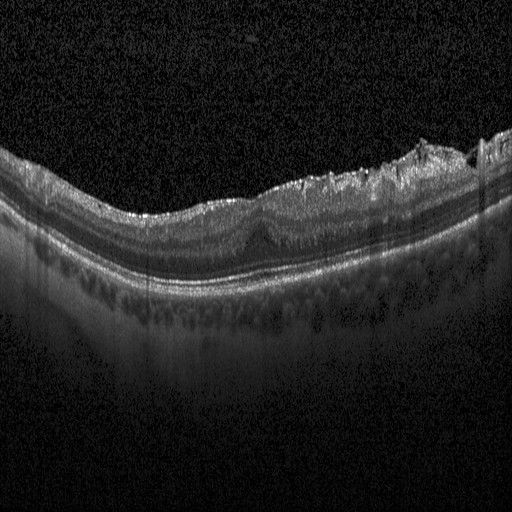 OCT finding: diabetic macular edema.